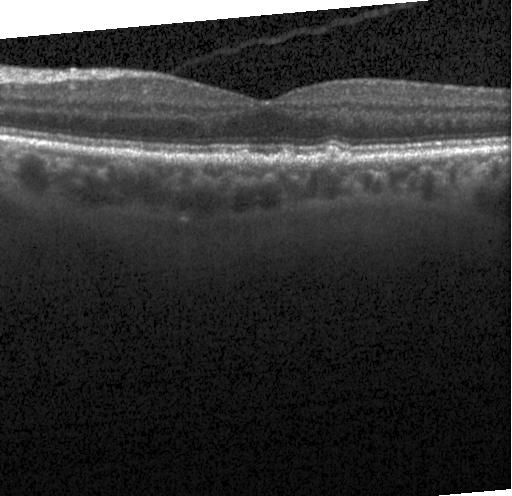

Spectral-domain optical coherence tomography, OCT line scan
Sub-RPE drusenoid deposits.